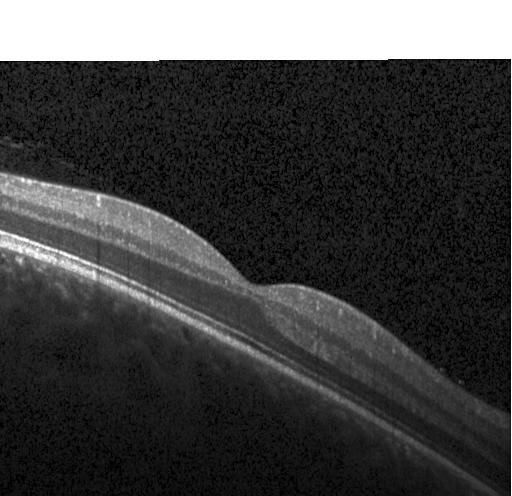 Diagnosis: no evidence of choroidal neovascularization, diabetic macular edema, or drusen.